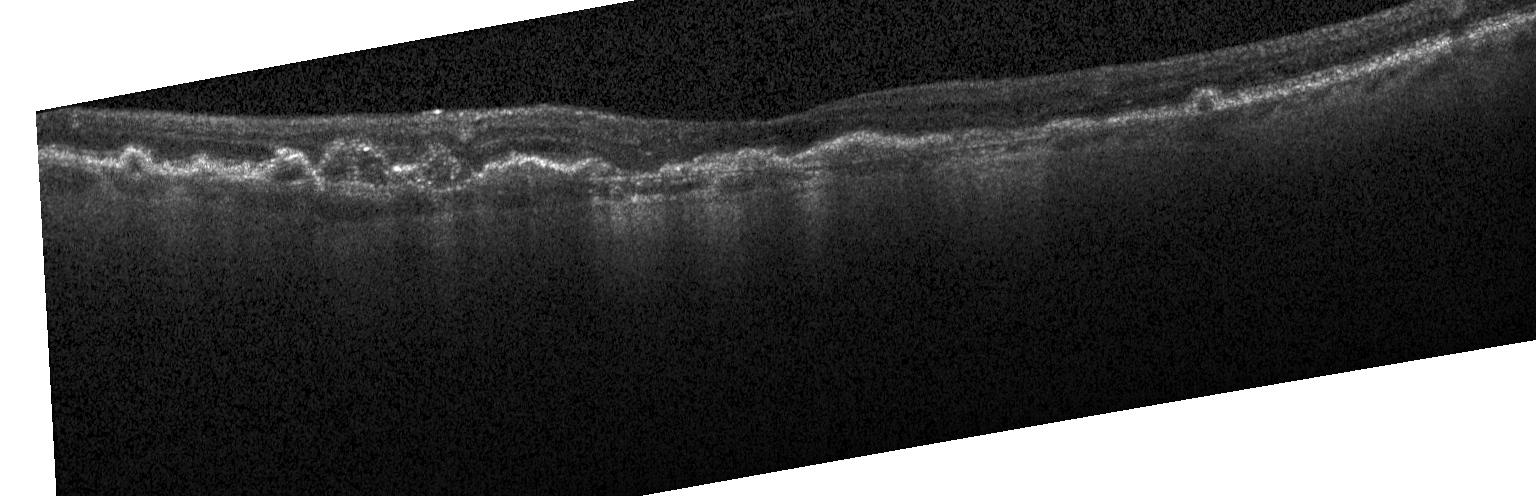 Retinal OCT cross-section showing CNV.